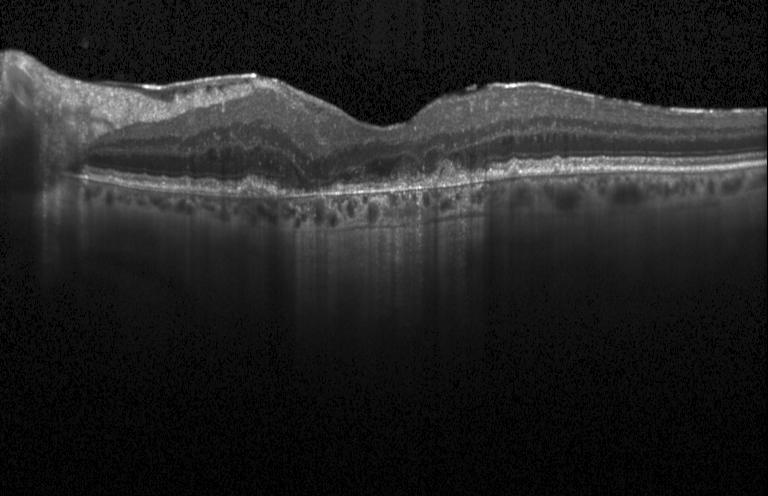

Optical coherence tomography B-scan. Through the macula — Impression: a choroidal neovascular membrane.